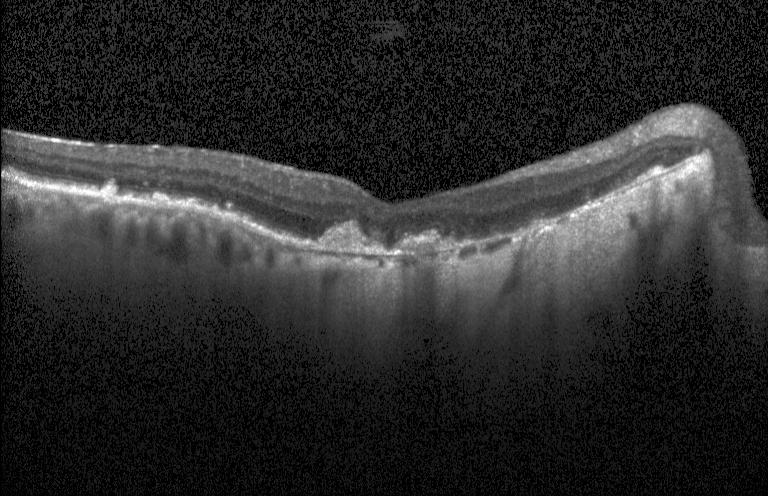

Spectral-domain optical coherence tomography. Retinal OCT B-scan. Acquired on a Heidelberg Spectralis. Through the macula. Impression: a choroidal neovascular membrane.